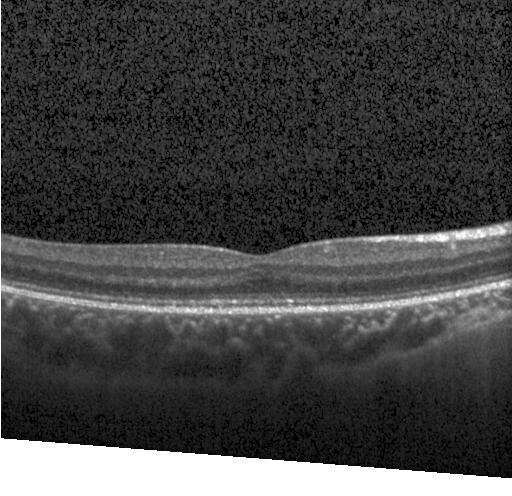

OCT line scan. The scan shows no choroidal neovascularization, no diabetic macular edema, and no drusen.